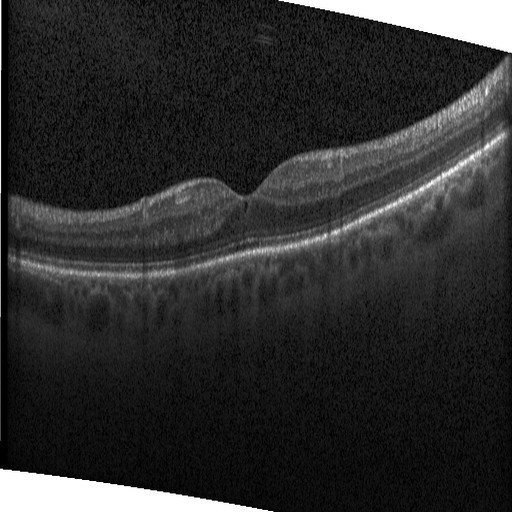 Spectral-domain OCT · optical coherence tomography scan · acquired on a Heidelberg Spectralis
The scan shows diabetic macular edema (DME).